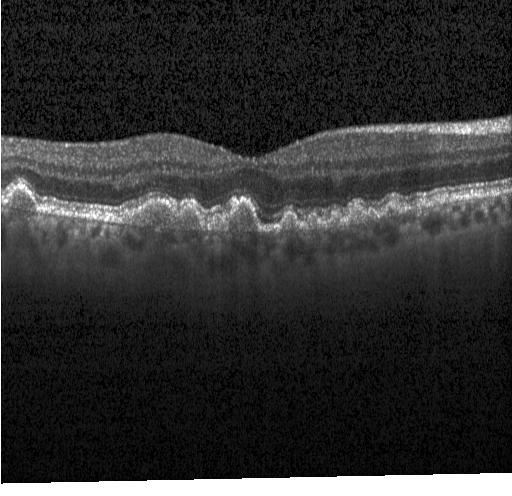 Centered on the fovea. OCT B-scan.
Finding: sub-RPE drusenoid deposits.